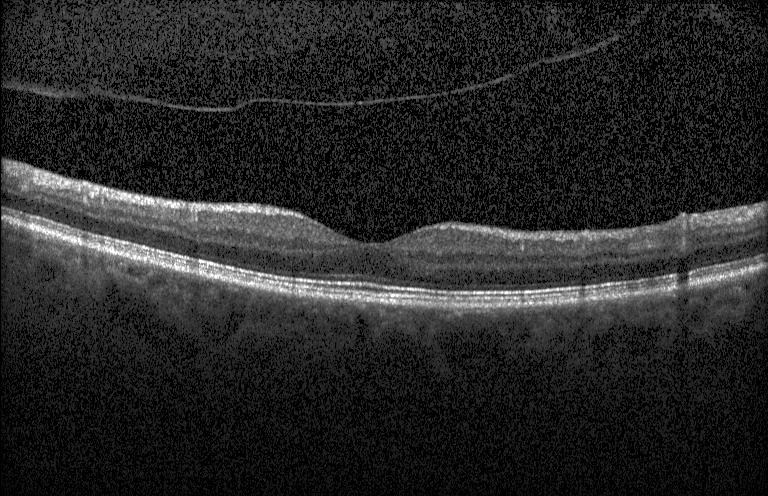
The scan shows neither choroidal neovascularization, diabetic macular edema, nor drusen.